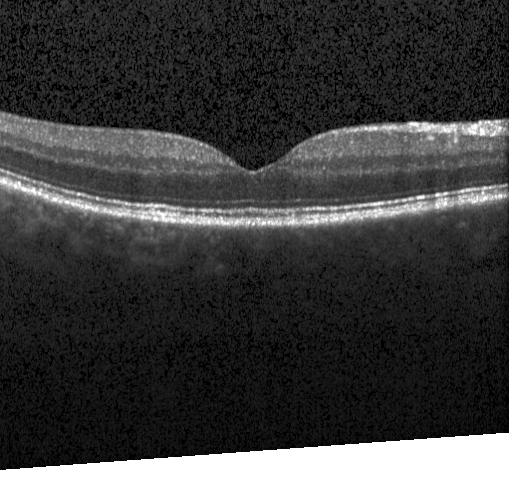

Heidelberg Spectralis OCT system. Optical coherence tomography scan. Spectral-domain OCT. Through the macula. This B-scan demonstrates no CNV, DME, or drusen.